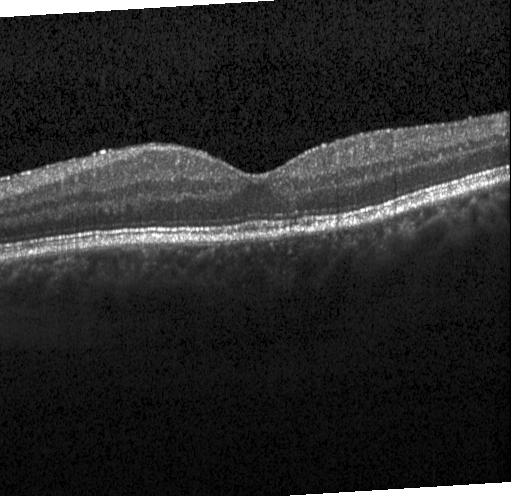
Spectral-domain OCT, centered on the fovea, acquired on a Heidelberg Spectralis, optical coherence tomography scan.
Finding: no choroidal neovascularization, no diabetic macular edema, and no drusen.